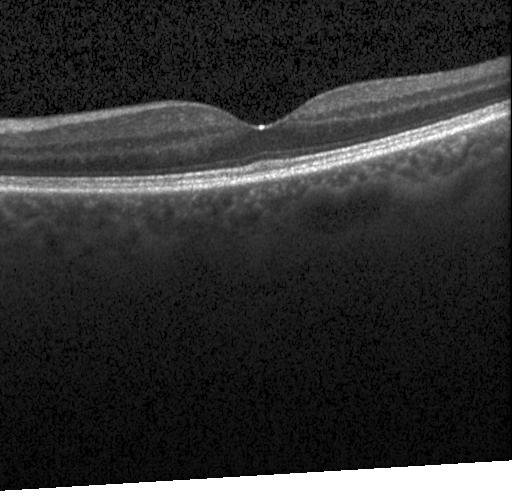
Optical coherence tomography B-scan, centered on the fovea — No CNV, no DME, and no drusen.